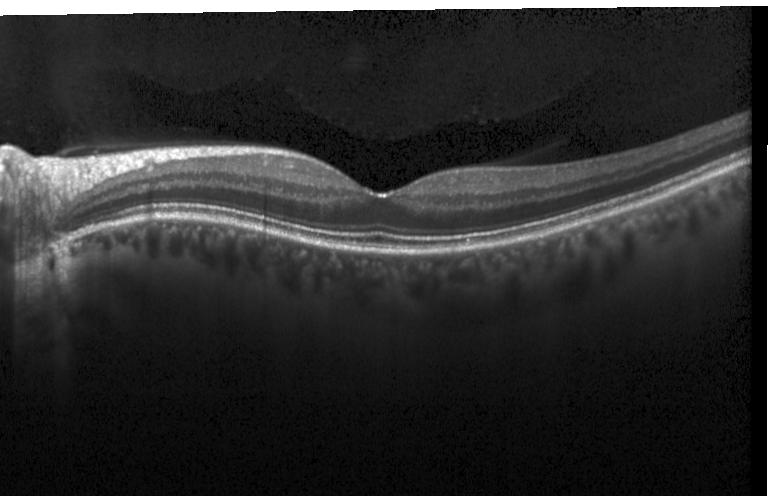 Acquired on a Heidelberg Spectralis · spectral-domain OCT · horizontal scan through the fovea · OCT B-scan. Neither CNV, DME, nor drusen.